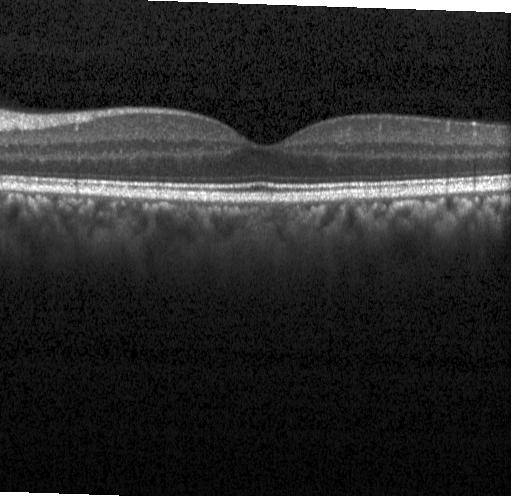
Spectral-domain OCT. Through the macula. Optical coherence tomography B-scan. Instrument: Heidelberg Spectralis
Macular OCT: no evidence of CNV, DME, or drusen.